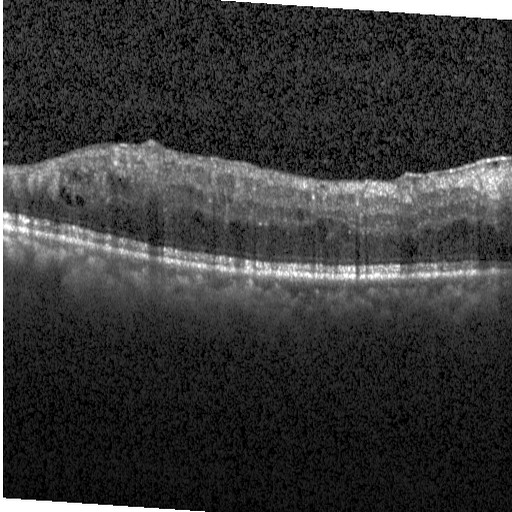 SD-OCT; acquired on a Heidelberg Spectralis; OCT B-scan; through the macula — OCT finding: diabetic macular edema.